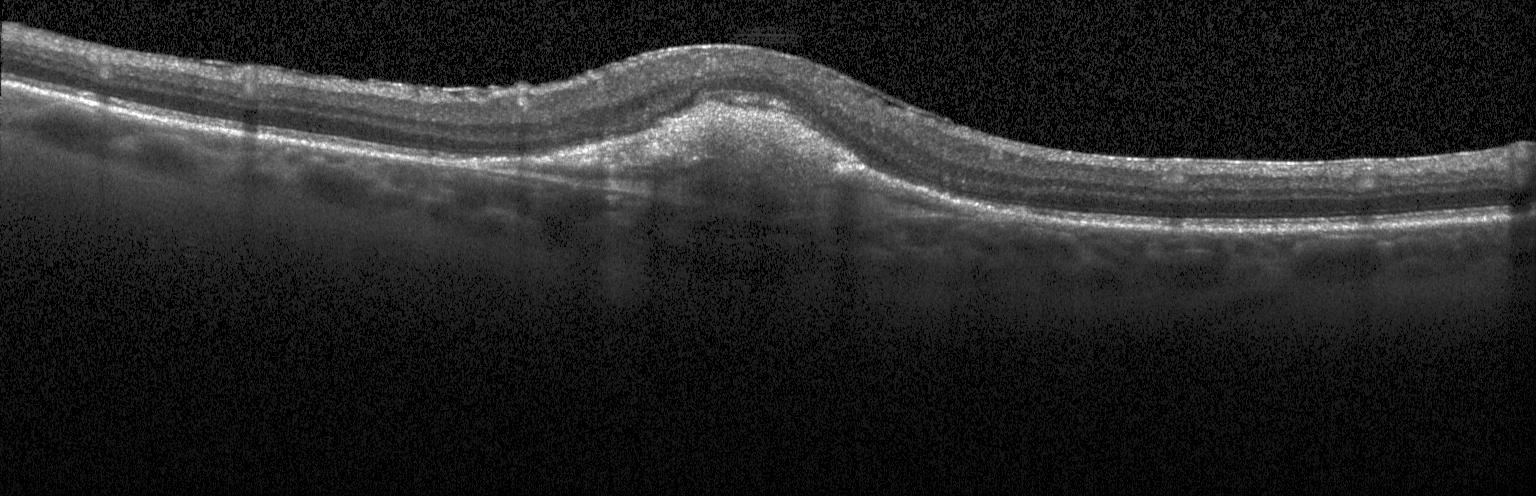
Retinal OCT B-scan; centered on the fovea; SD-OCT — This B-scan demonstrates a choroidal neovascular membrane.